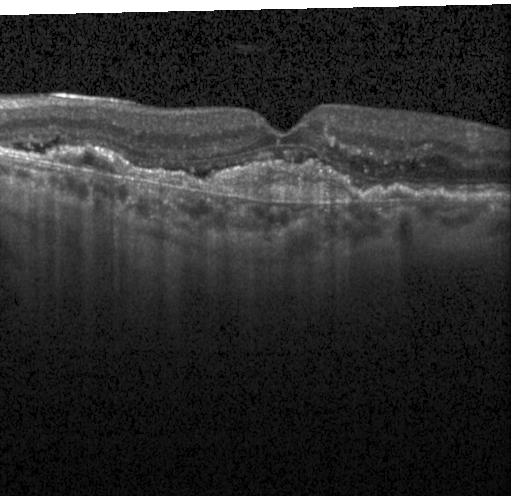

Finding: CNV.